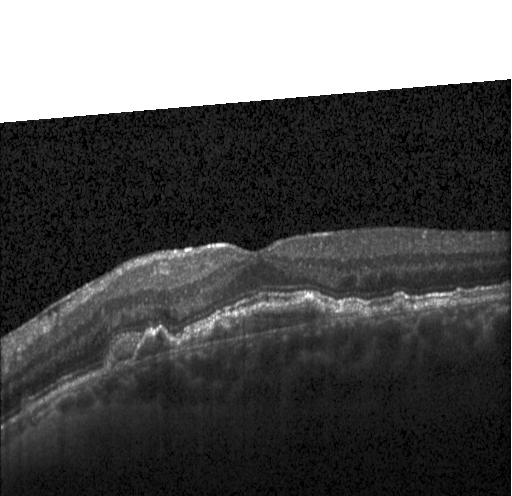
Spectral-domain optical coherence tomography; Heidelberg Spectralis OCT system; optical coherence tomography scan — Finding: CNV.